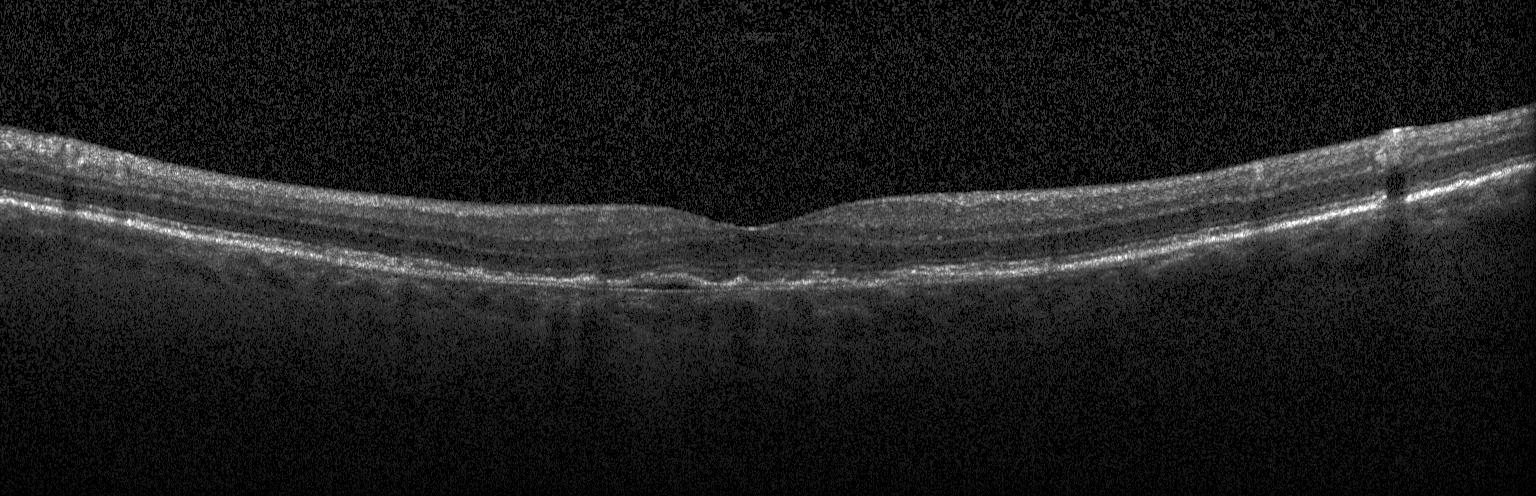
OCT scan showing a choroidal neovascular membrane.